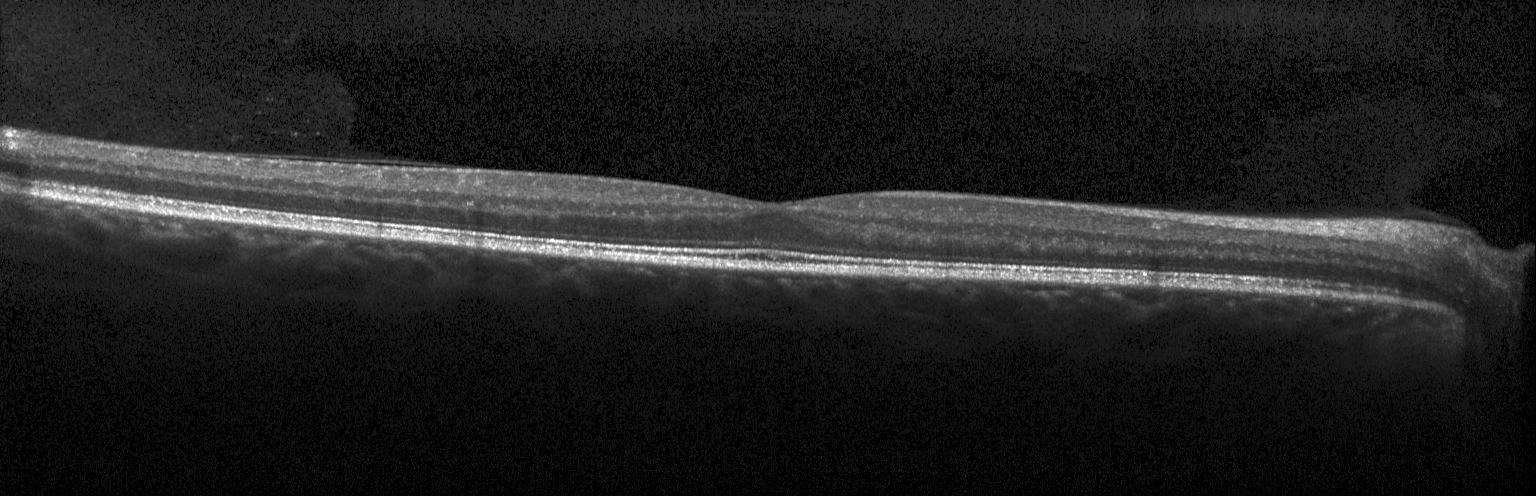

Optical coherence tomography B-scan. Spectral-domain optical coherence tomography
Diagnosis: no choroidal neovascularization, diabetic macular edema, or drusen.